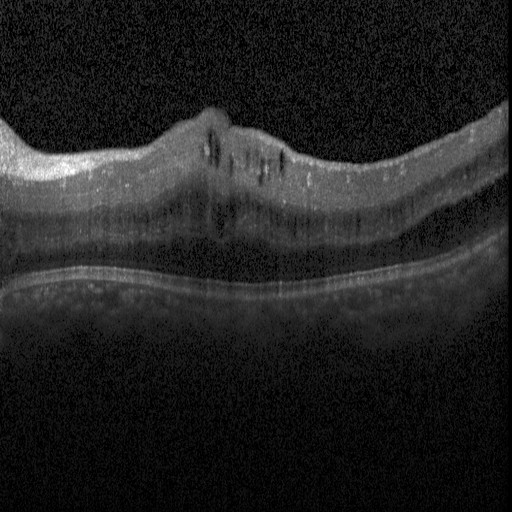 OCT B-scan.
Diagnosis: DME.